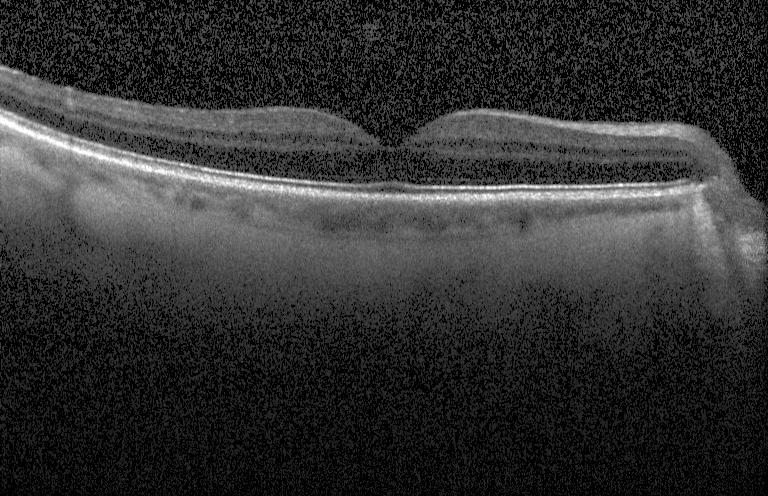
Heidelberg Spectralis OCT system. Horizontal scan through the fovea. SD-OCT. Retinal OCT cross-section — Finding: no choroidal neovascularization, no diabetic macular edema, and no drusen.